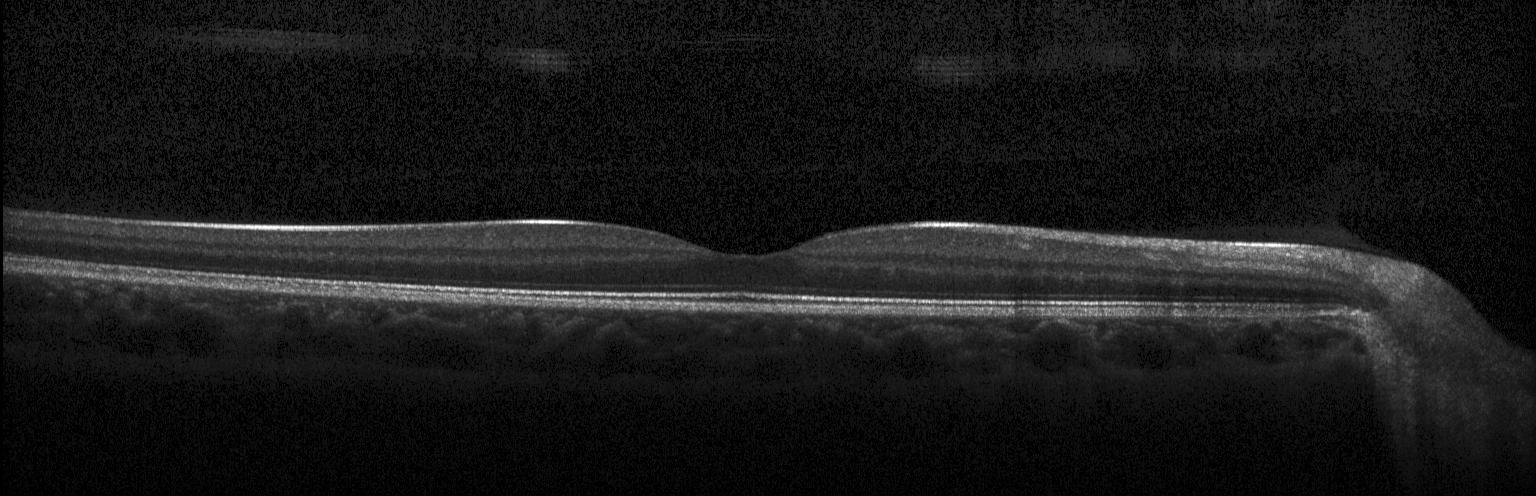 OCT line scan; SD-OCT; horizontal scan through the fovea; Heidelberg Spectralis.
Finding: no choroidal neovascularization, diabetic macular edema, or drusen.